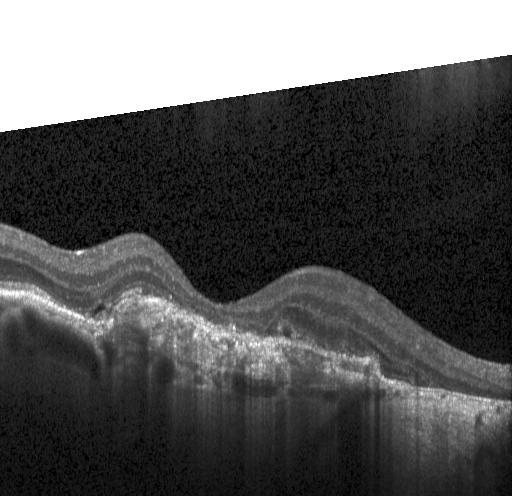

Heidelberg Spectralis OCT system, spectral-domain OCT, macular scan, retinal OCT cross-section — Impression: a choroidal neovascular membrane.